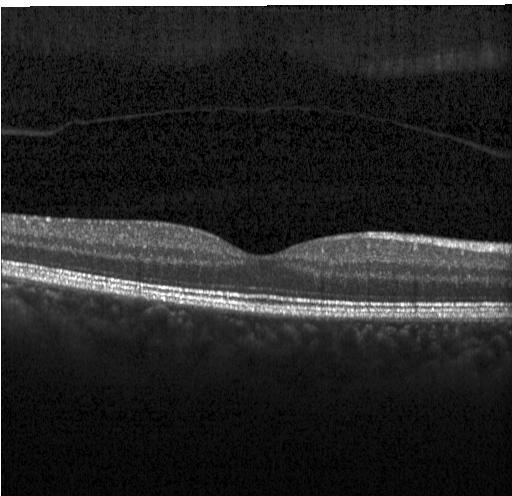

OCT B-scan.
Finding: no evidence of choroidal neovascularization, diabetic macular edema, or drusen.